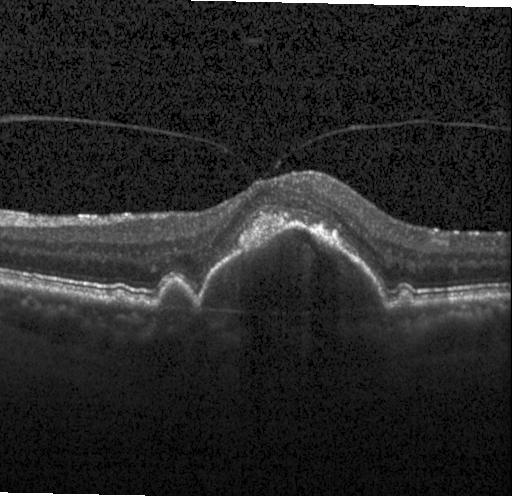
Optical coherence tomography scan — The scan shows choroidal neovascularization (CNV).